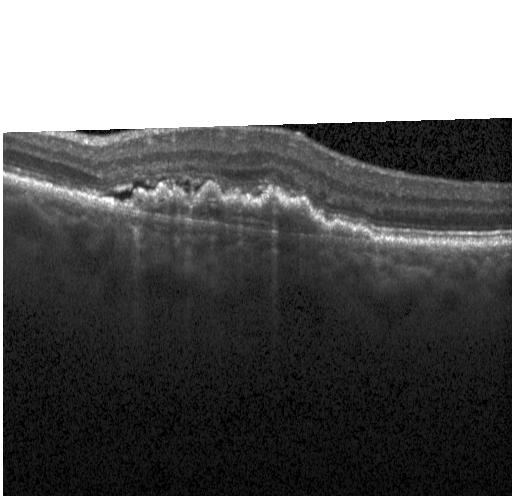
Assessment: a choroidal neovascular membrane.